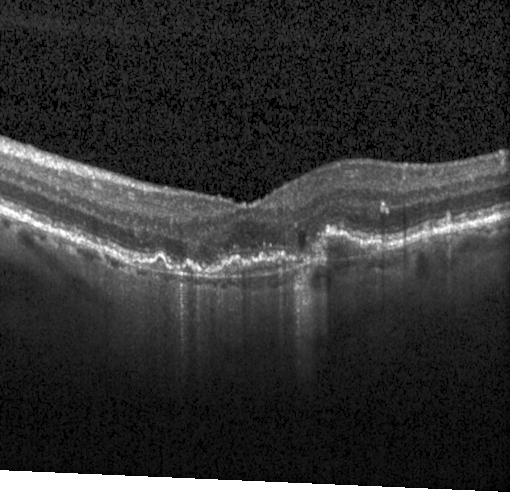 Heidelberg Spectralis, optical coherence tomography B-scan. Choroidal neovascularization (CNV).